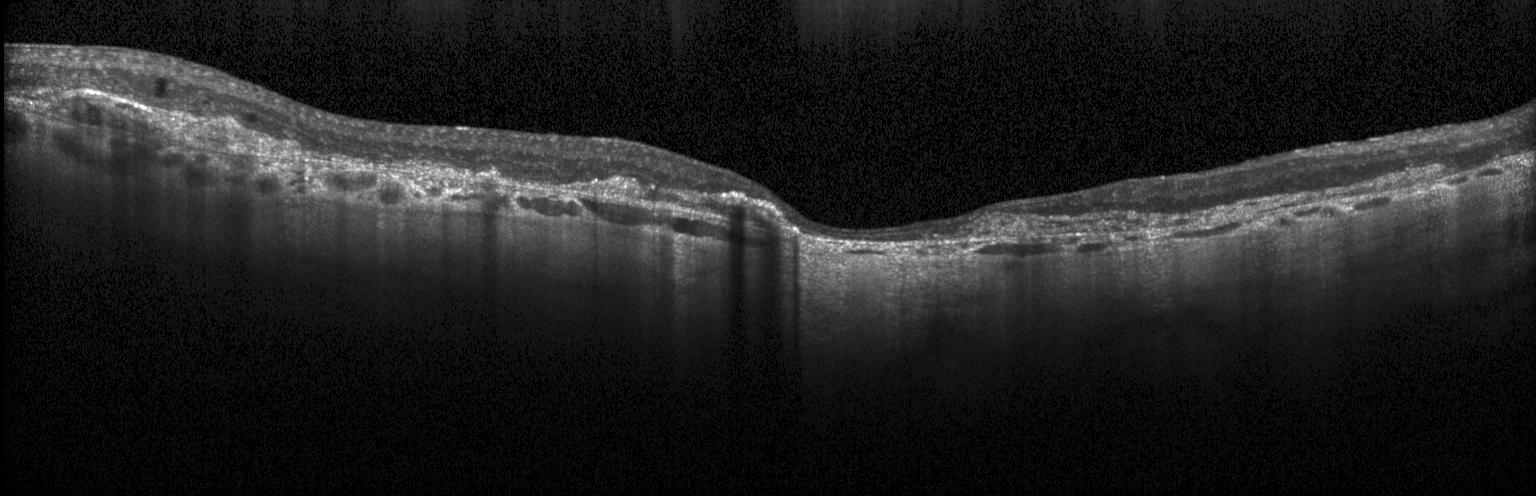
Spectral-domain optical coherence tomography, Heidelberg Spectralis, optical coherence tomography scan
Finding: choroidal neovascularization.